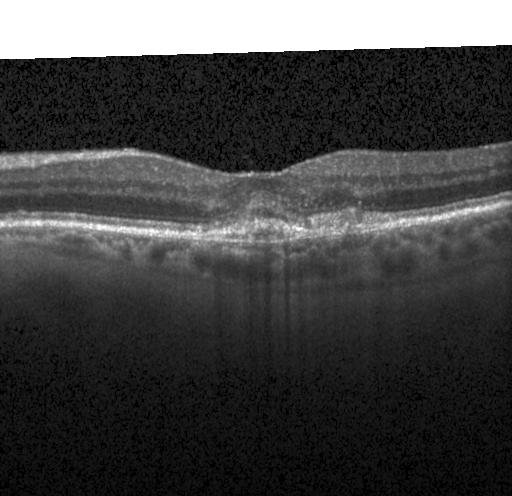

Retinal OCT cross-section
Diagnosis: a choroidal neovascular membrane.